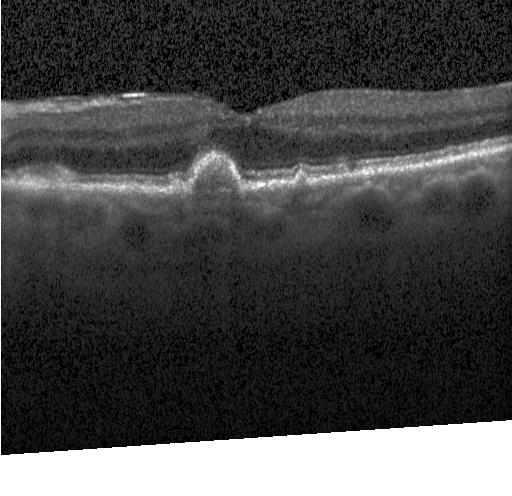
OCT B-scan. Multiple drusen.